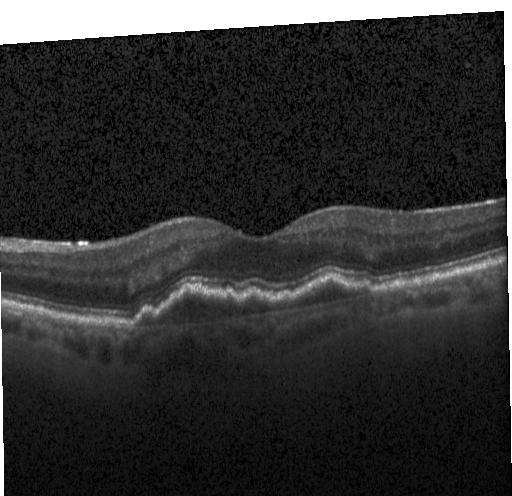

SD-OCT. Retinal OCT cross-section. Heidelberg Spectralis OCT system — OCT finding: a choroidal neovascular membrane.